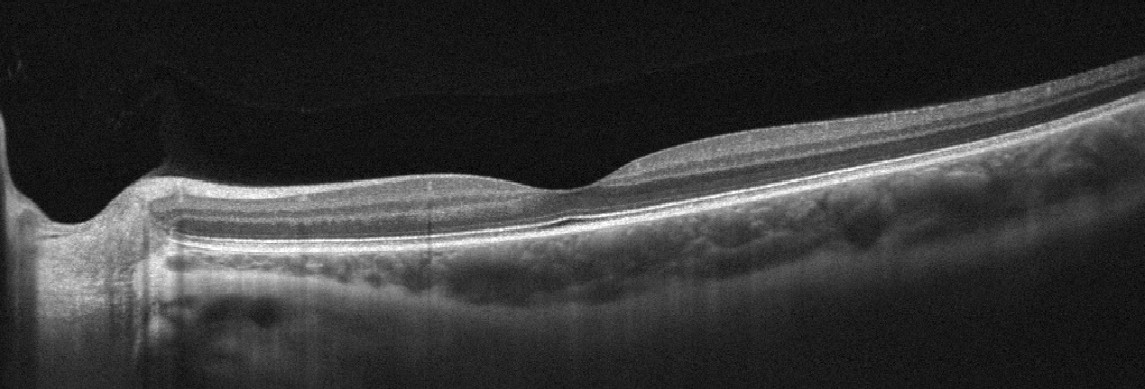
Macular scan, Optovue Avanti RTVue XR, optical coherence tomography scan. OCT finding: absence of AMD, DME, ERM, RAO, RVO, and vitreomacular interface disease.